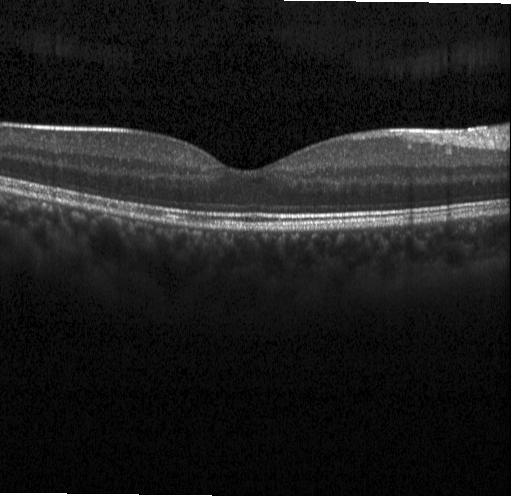 OCT line scan.
Macular OCT: no CNV, DME, or drusen.